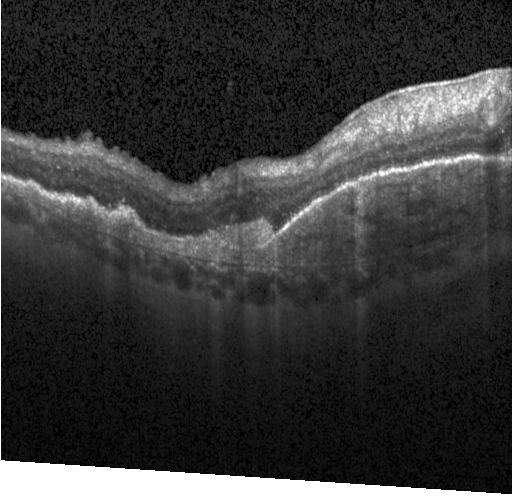 Retinal OCT cross-section
Impression: a choroidal neovascular membrane.